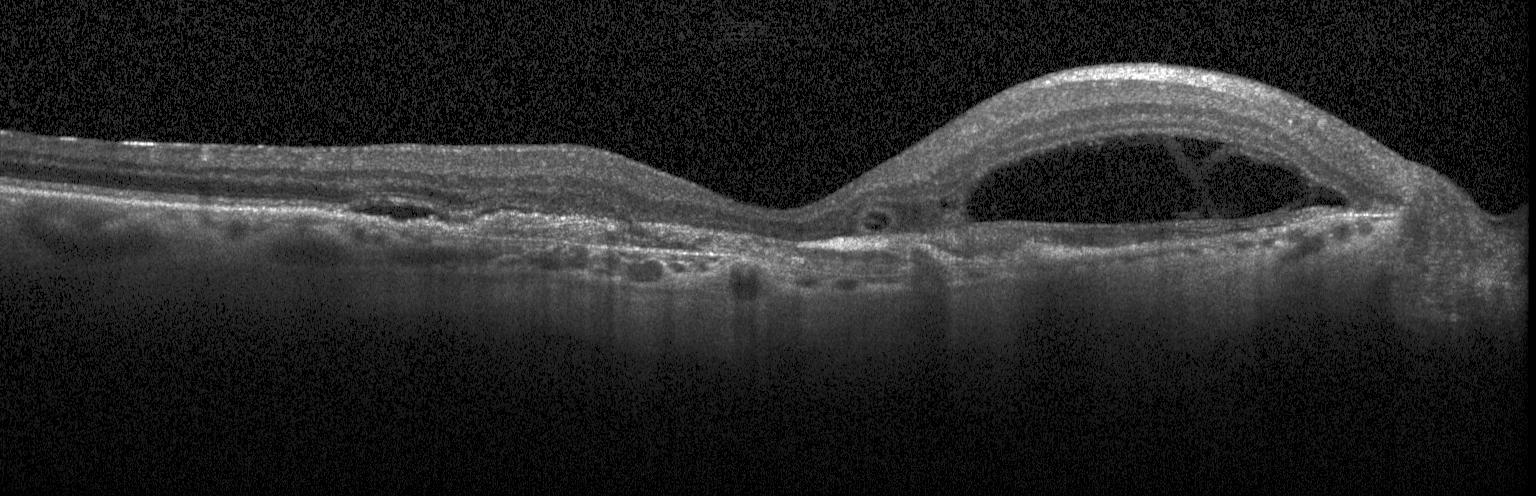
The scan shows choroidal neovascularization (CNV).